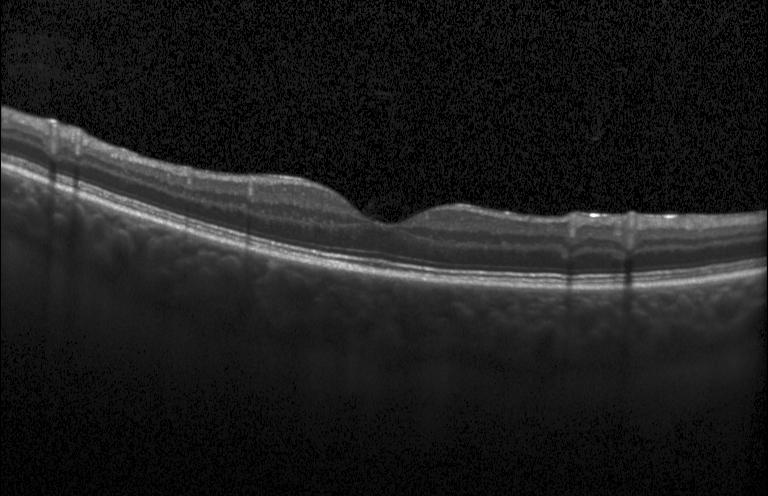

Spectral-domain OCT B-scan: no CNV, no DME, and no drusen.